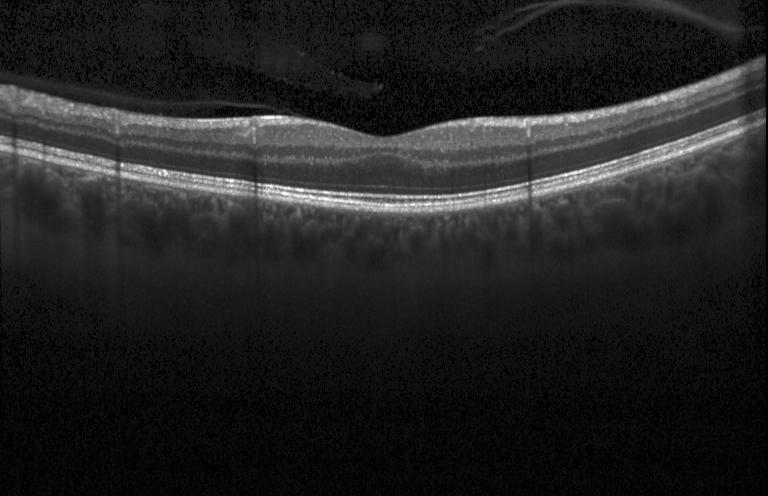 Heidelberg Spectralis OCT system, spectral-domain optical coherence tomography, OCT line scan, fovea-centered — Impression: no evidence of choroidal neovascularization, diabetic macular edema, or drusen.